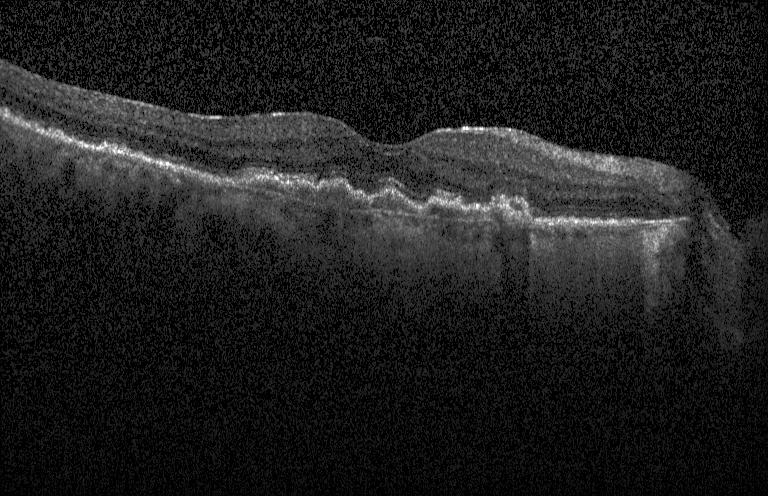
OCT B-scan · acquired on a Heidelberg Spectralis
Impression: a choroidal neovascular membrane.